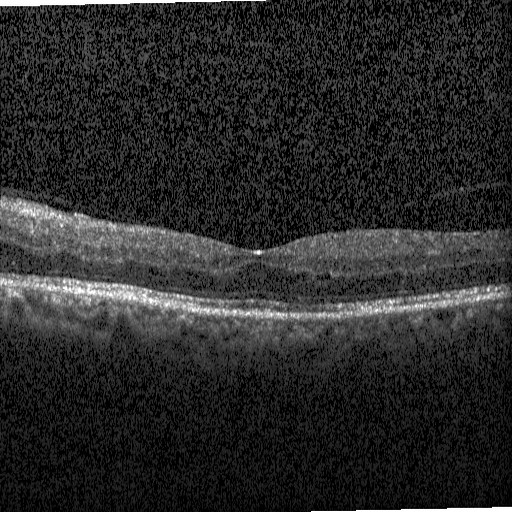 The scan shows diabetic macular edema (DME).